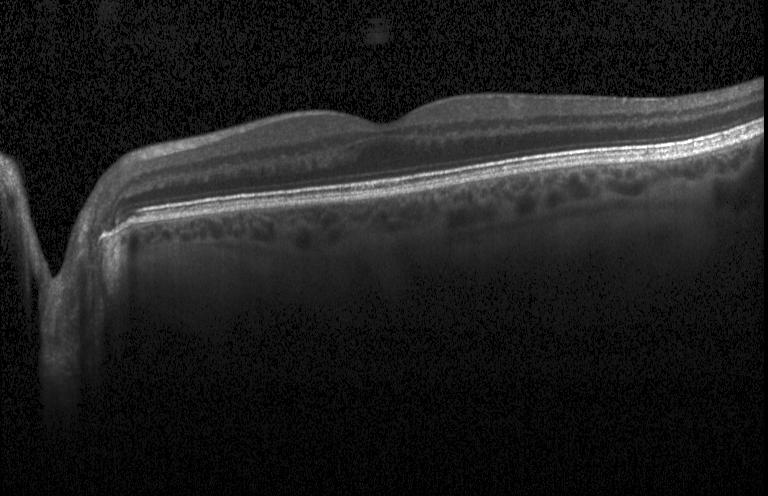

Macular OCT: no choroidal neovascularization, no diabetic macular edema, and no drusen.